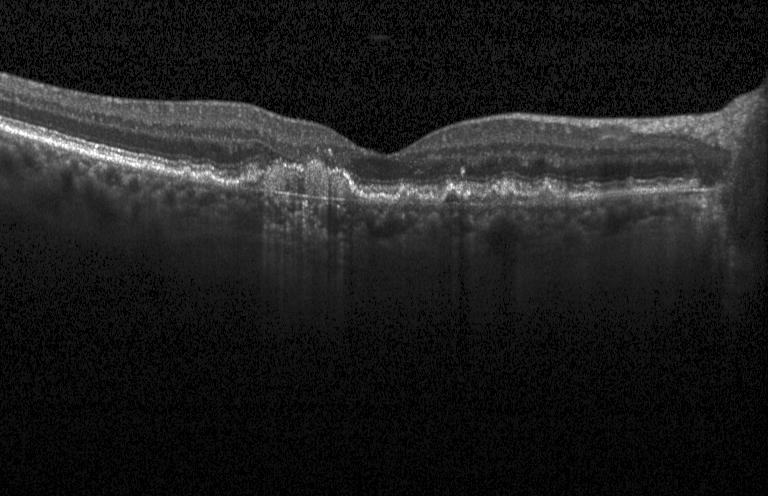 Impression: CNV.